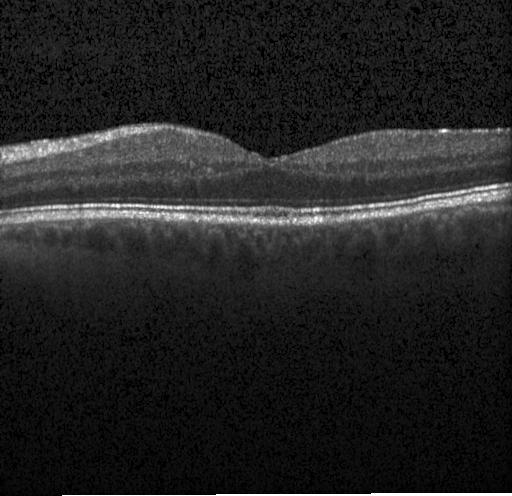
Retinal OCT cross-section showing neither choroidal neovascularization, diabetic macular edema, nor drusen.